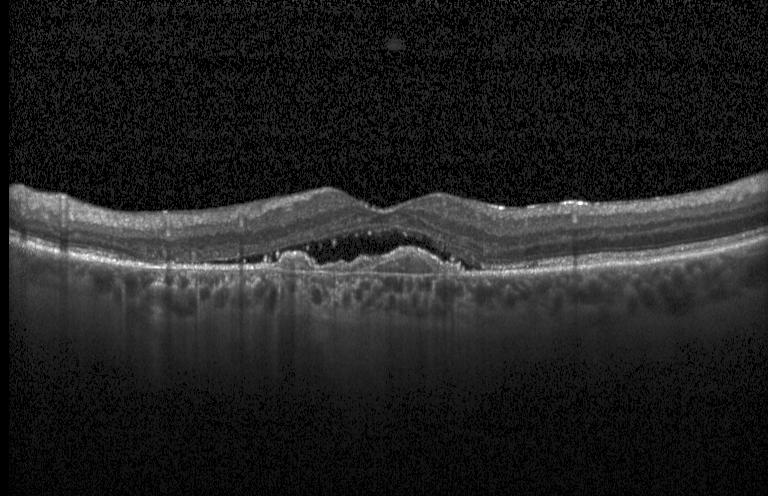 Optical coherence tomography scan. Heidelberg Spectralis. Finding: choroidal neovascularization.